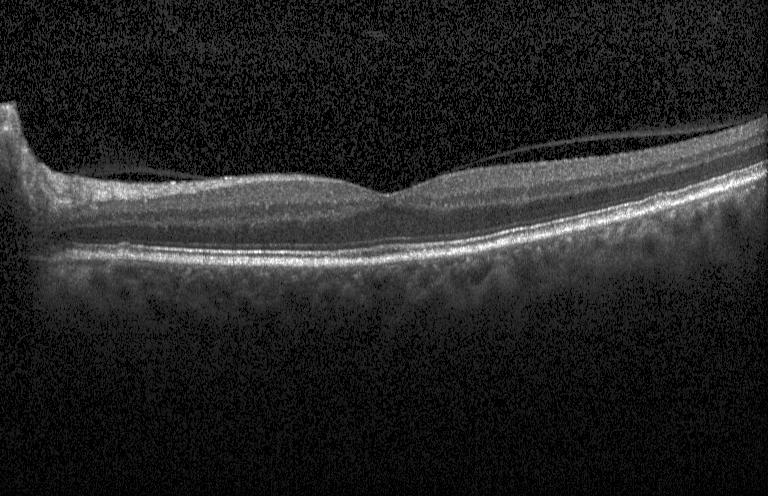
Heidelberg Spectralis OCT system. Fovea-centered. OCT B-scan. OCT finding: neither CNV, DME, nor drusen.